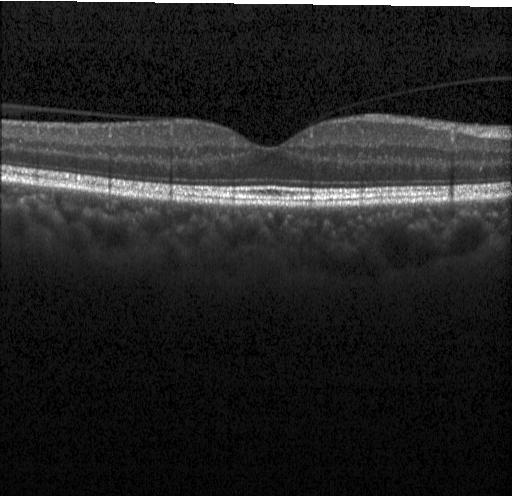 Spectral-domain OCT · centered on the fovea · OCT B-scan · Heidelberg Spectralis OCT system
No choroidal neovascularization, diabetic macular edema, or drusen.